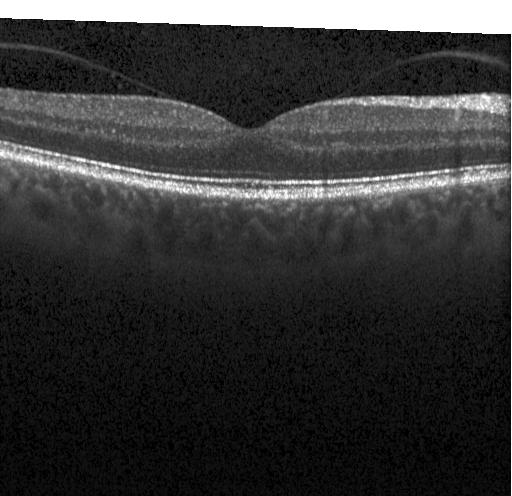
Diagnosis: neither CNV, DME, nor drusen.